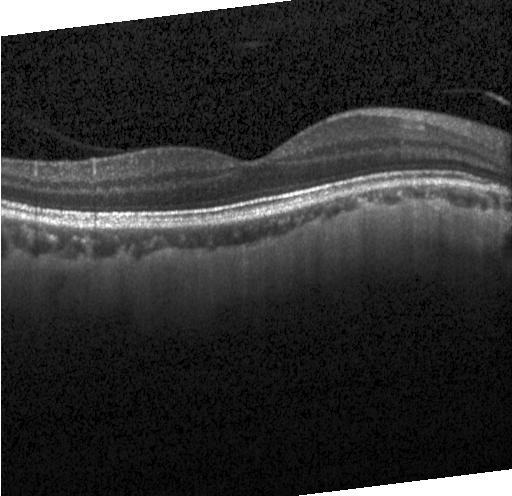 Spectral-domain OCT · optical coherence tomography scan · fovea-centered · instrument: Heidelberg Spectralis.
No choroidal neovascularization, diabetic macular edema, or drusen.